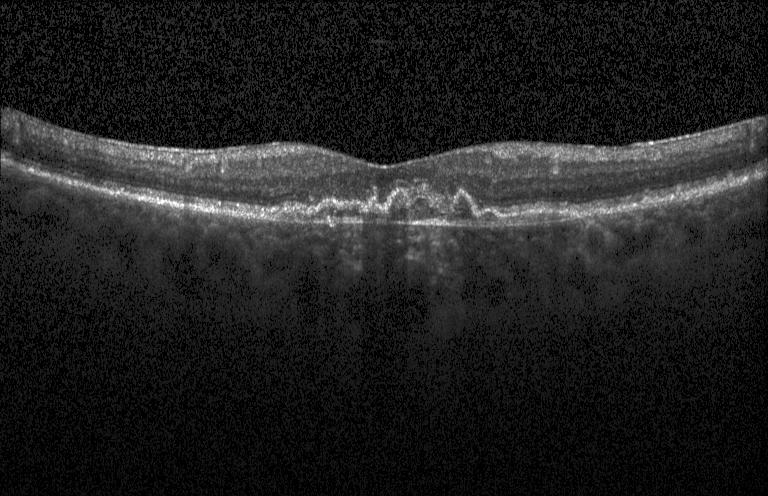

Heidelberg Spectralis · macular scan · OCT B-scan · SD-OCT.
This B-scan demonstrates a choroidal neovascular membrane.